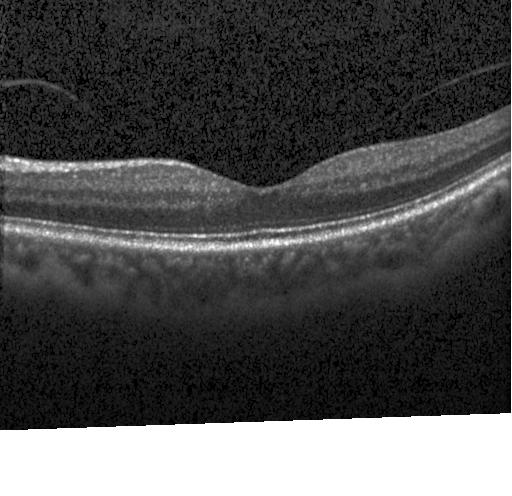

Retinal OCT cross-section. SD-OCT. Acquired on a Heidelberg Spectralis
Finding: no choroidal neovascularization, no diabetic macular edema, and no drusen.